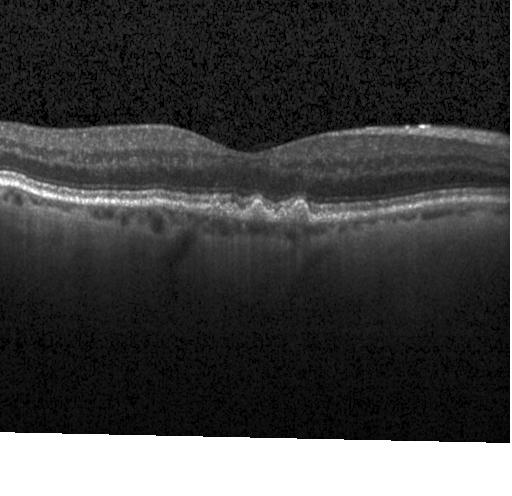

Retinal OCT cross-section.
Dx: drusen.